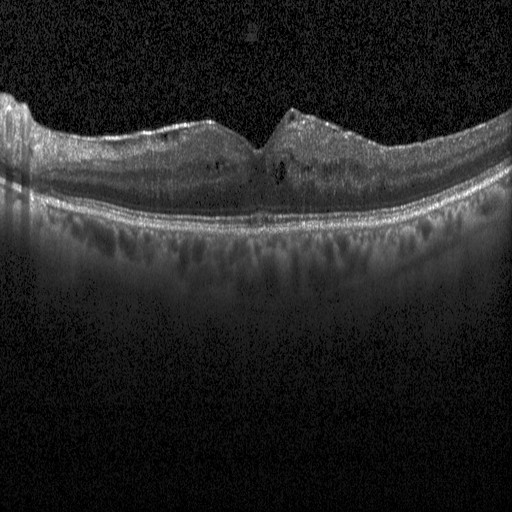
This B-scan demonstrates diabetic macular edema.